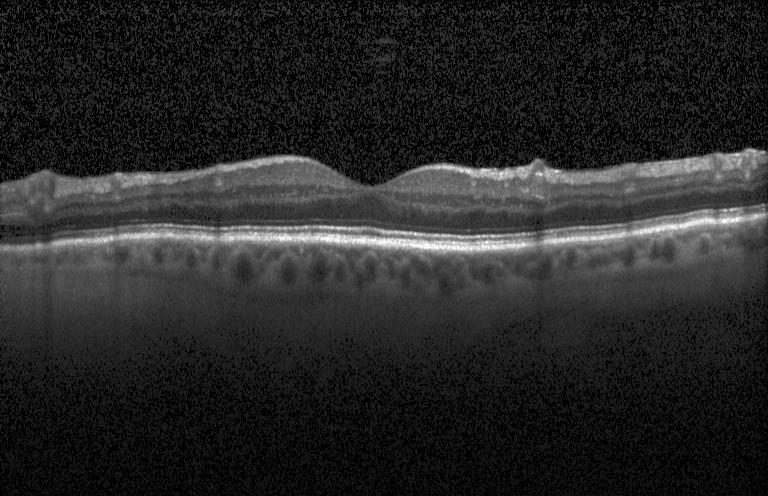 Spectral-domain optical coherence tomography. Retinal OCT B-scan — Diagnosis: no choroidal neovascularization, diabetic macular edema, or drusen.